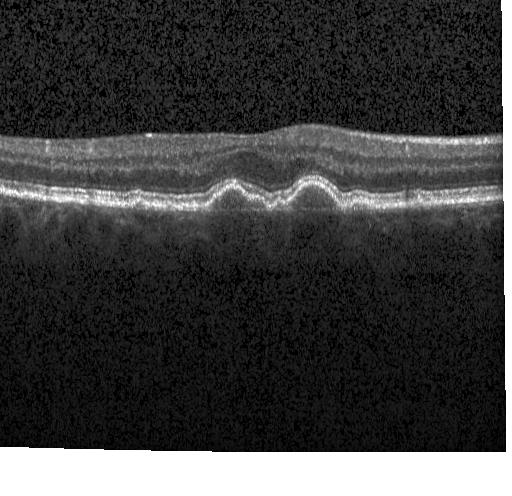

Centered on the fovea. OCT B-scan. This B-scan demonstrates drusen.